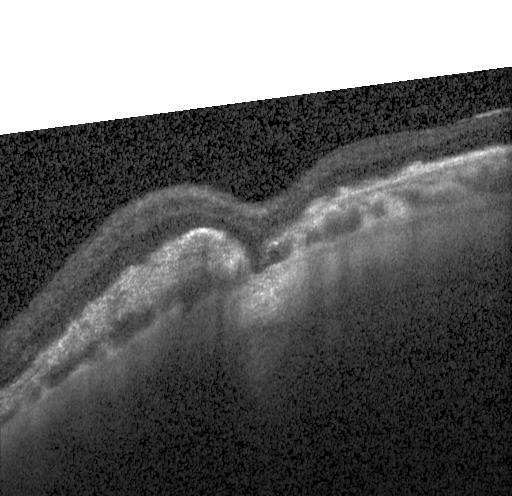

Optical coherence tomography scan · Heidelberg Spectralis · SD-OCT
Macular OCT: a choroidal neovascular membrane.